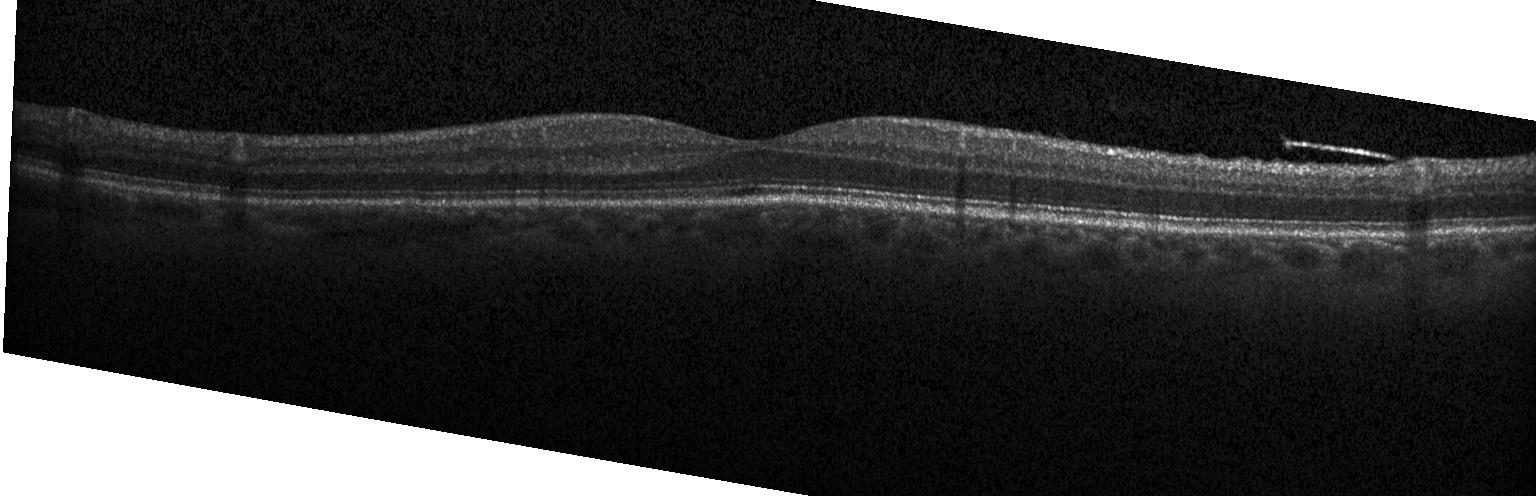

Impression: no CNV, no DME, and no drusen.